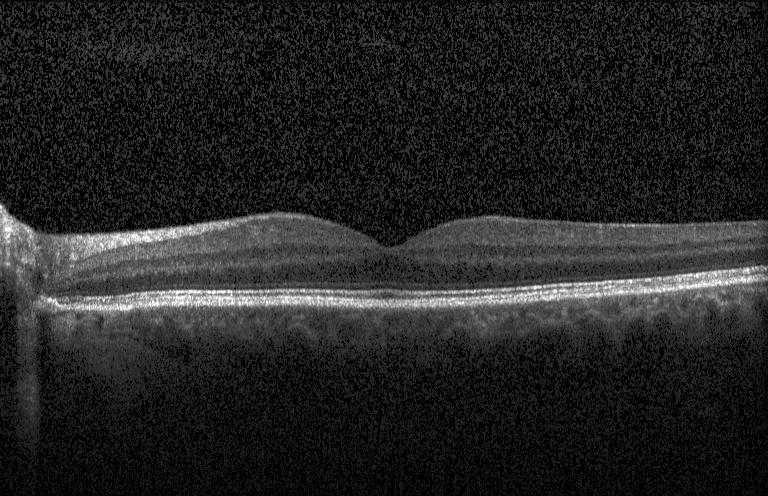 Heidelberg Spectralis, retinal OCT cross-section
Diagnosis: no choroidal neovascularization, no diabetic macular edema, and no drusen.